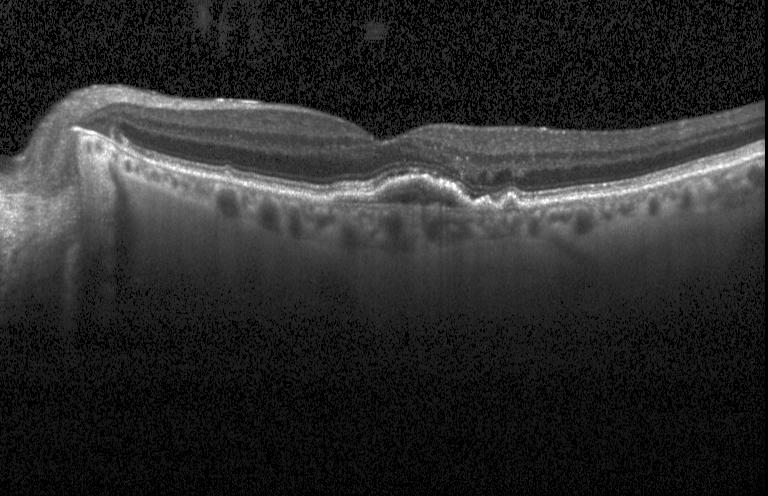

OCT finding: CNV.